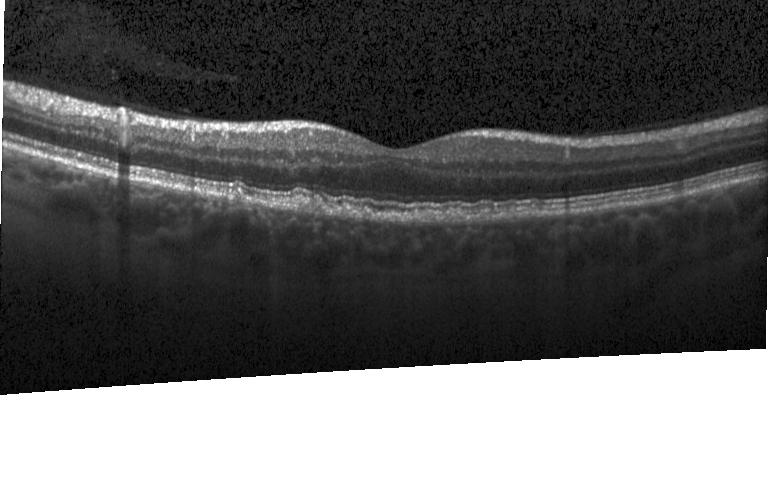
OCT B-scan showing sub-RPE drusenoid deposits.